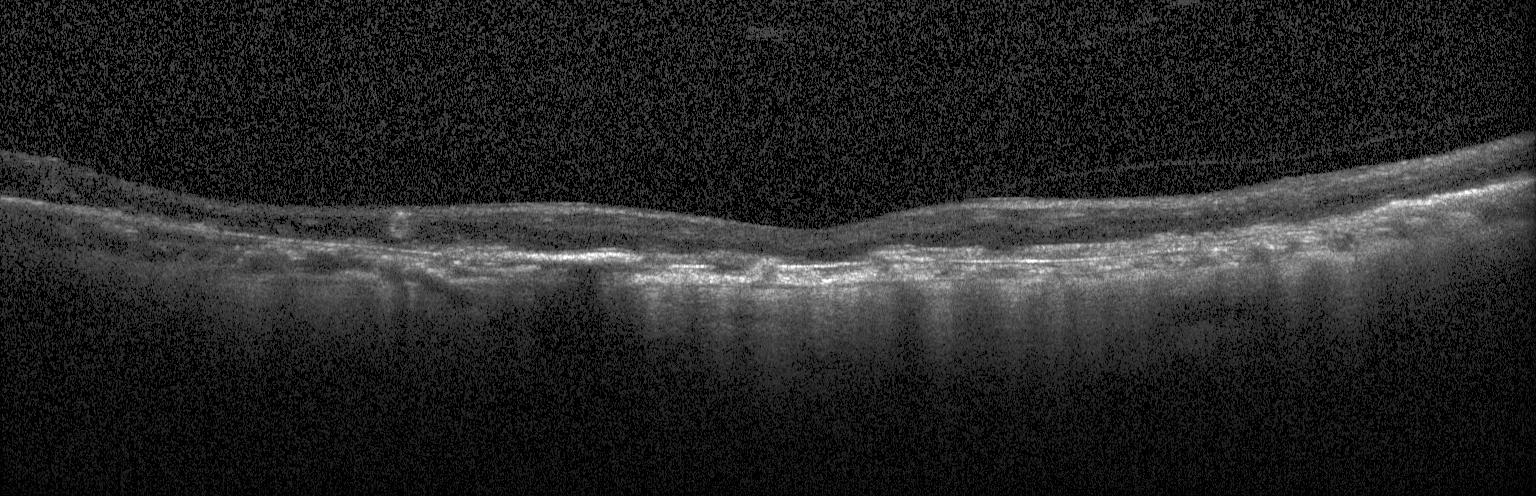
Acquired on a Heidelberg Spectralis; through the macula; OCT B-scan; spectral-domain optical coherence tomography — OCT finding: a choroidal neovascular membrane.